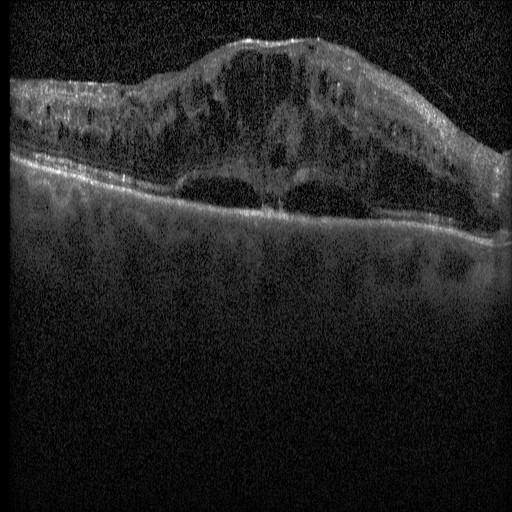
Impression: DME.